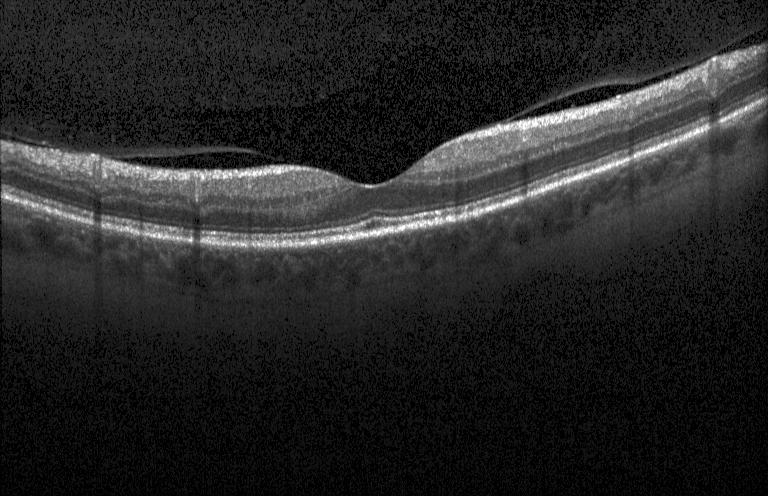

Spectral-domain OCT · OCT line scan. Assessment: no choroidal neovascularization, diabetic macular edema, or drusen.